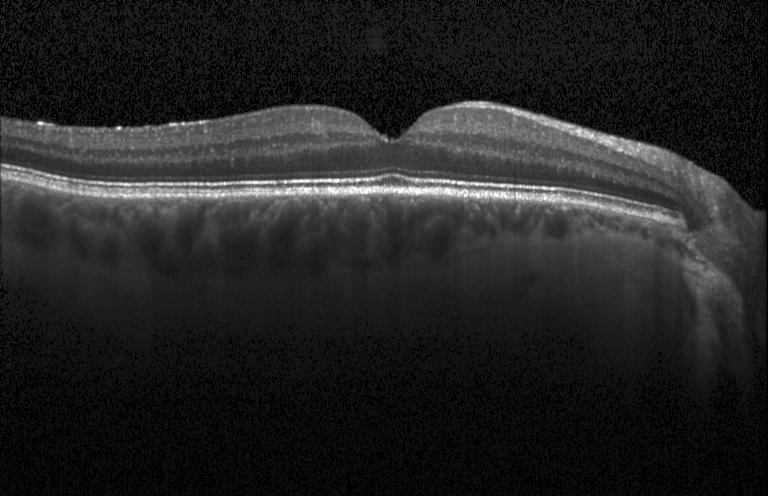 No CNV, no DME, and no drusen.